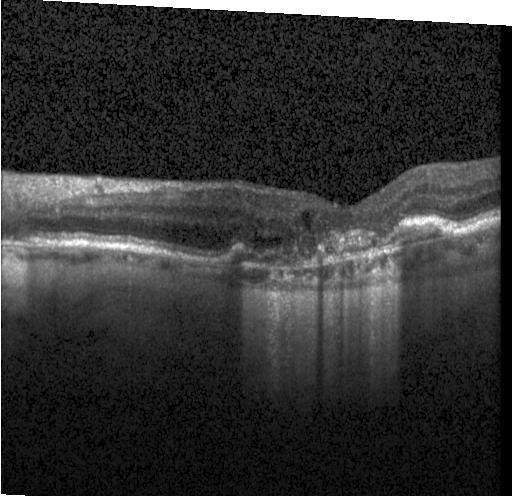
Finding: a choroidal neovascular membrane.